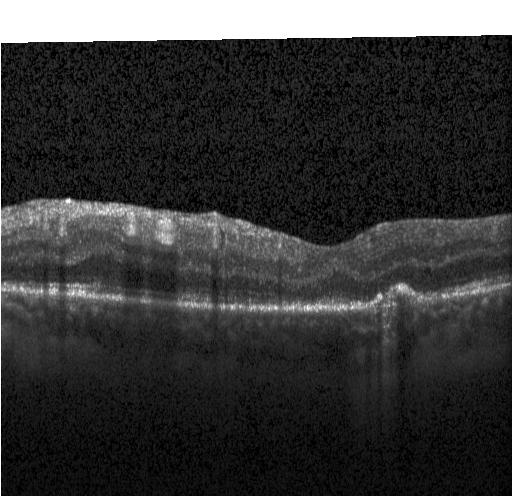 OCT B-scan.
Finding: a choroidal neovascular membrane.